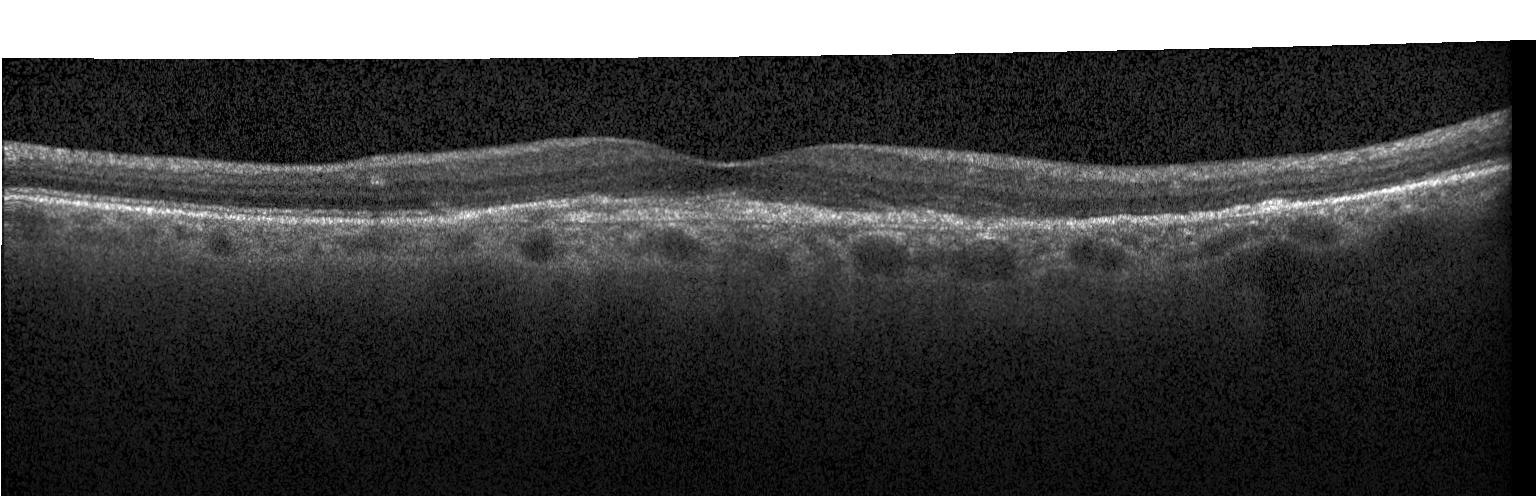
OCT B-scan
Diagnosis: choroidal neovascularization.